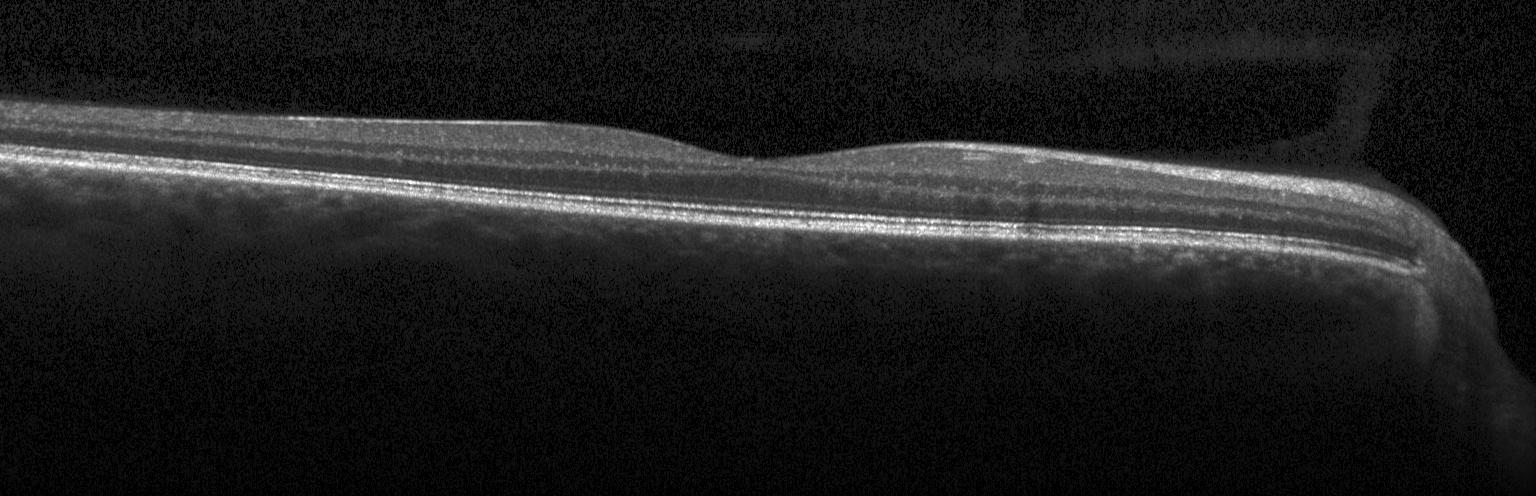
OCT B-scan showing no choroidal neovascularization, no diabetic macular edema, and no drusen.